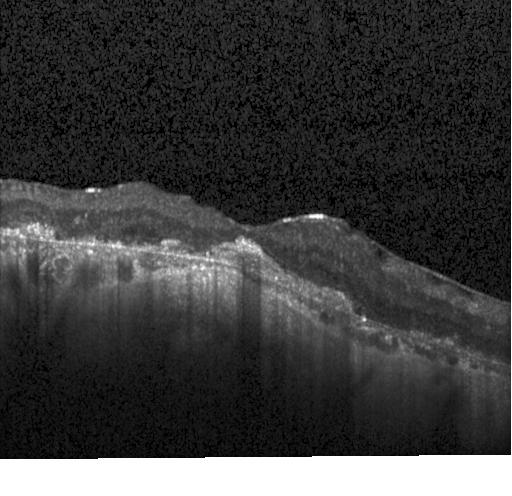

Heidelberg Spectralis OCT system, spectral-domain OCT, macular scan, retinal OCT cross-section. Macular OCT: a choroidal neovascular membrane.